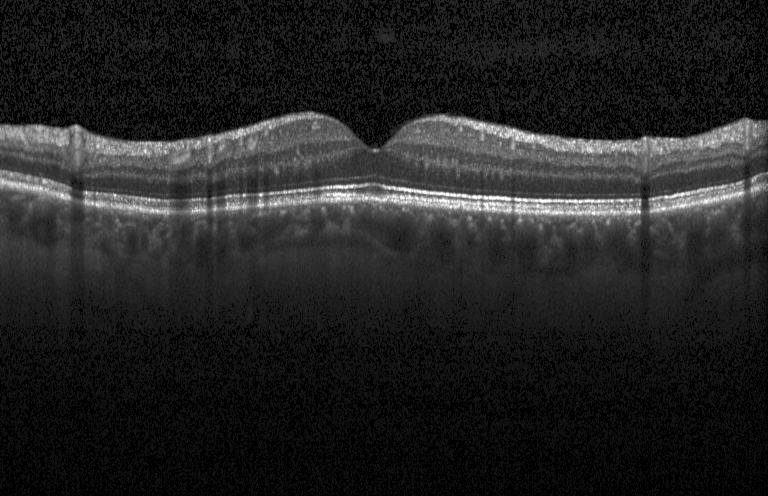

The scan shows neither CNV, DME, nor drusen.